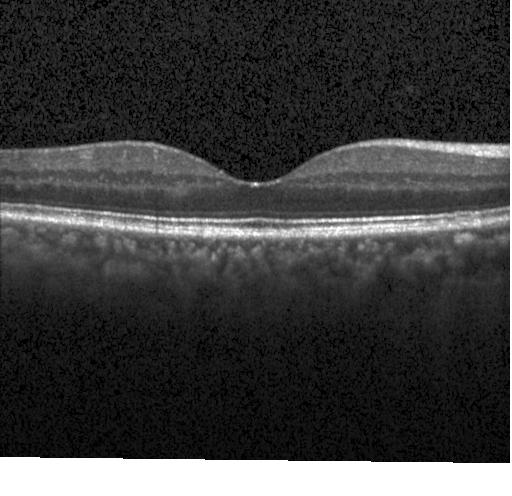
OCT B-scan. SD-OCT. Heidelberg Spectralis. Through the macula. Neither CNV, DME, nor drusen.